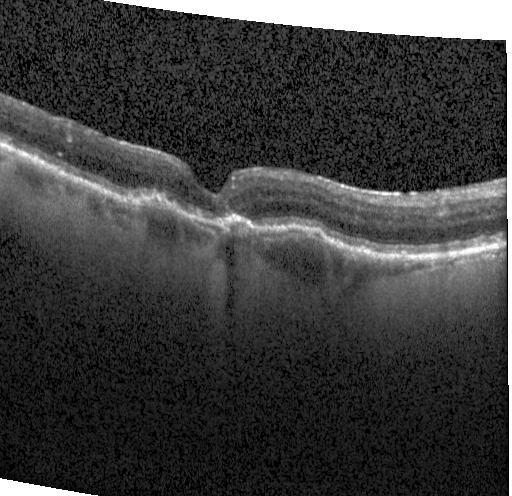 SD-OCT. Heidelberg Spectralis OCT system. OCT B-scan — Impression: choroidal neovascularization (CNV).